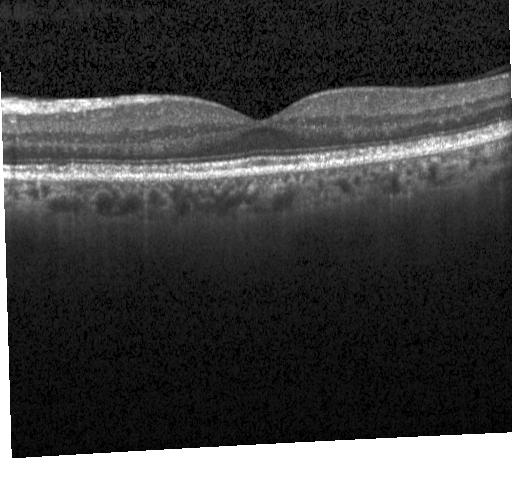
OCT B-scan · acquired on a Heidelberg Spectralis.
Dx: neither choroidal neovascularization, diabetic macular edema, nor drusen.